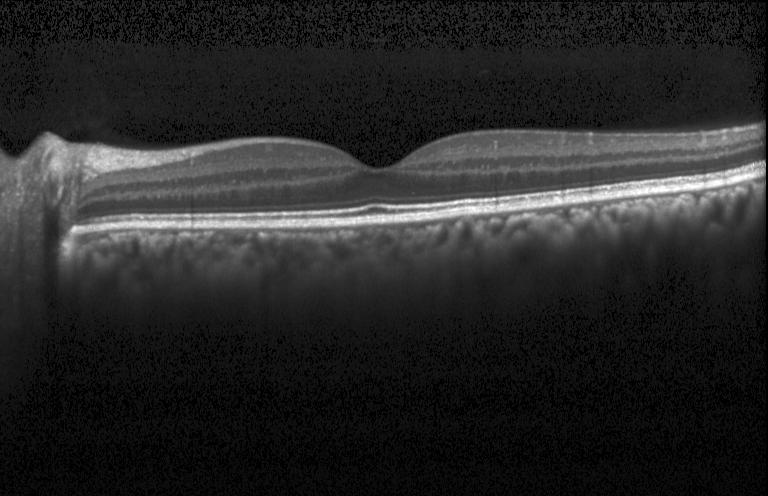
OCT B-scan — No choroidal neovascularization, diabetic macular edema, or drusen.